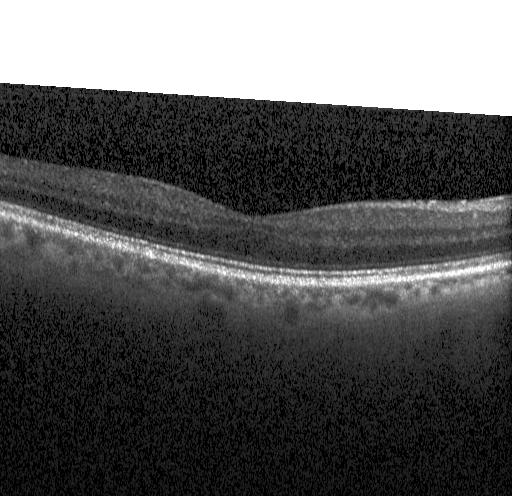

Spectral-domain optical coherence tomography. Acquired on a Heidelberg Spectralis. Retinal OCT B-scan. Horizontal scan through the fovea — Diagnosis: neither choroidal neovascularization, diabetic macular edema, nor drusen.